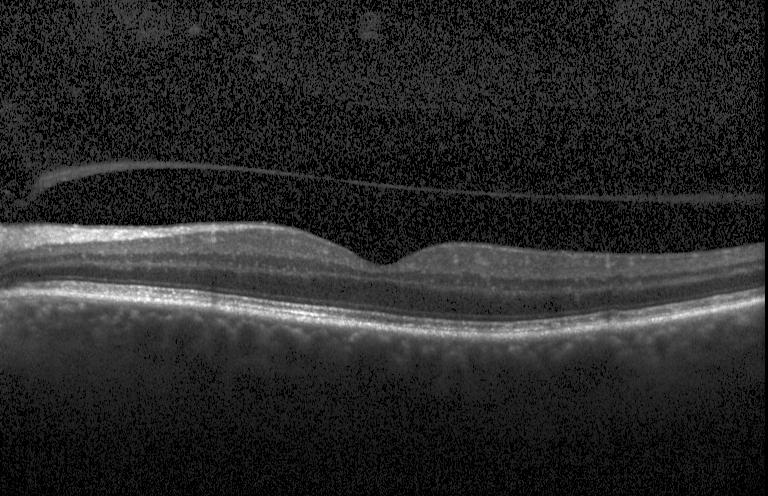
Through the macula · spectral-domain optical coherence tomography · Heidelberg Spectralis · optical coherence tomography B-scan.
Dx: no choroidal neovascularization, diabetic macular edema, or drusen.